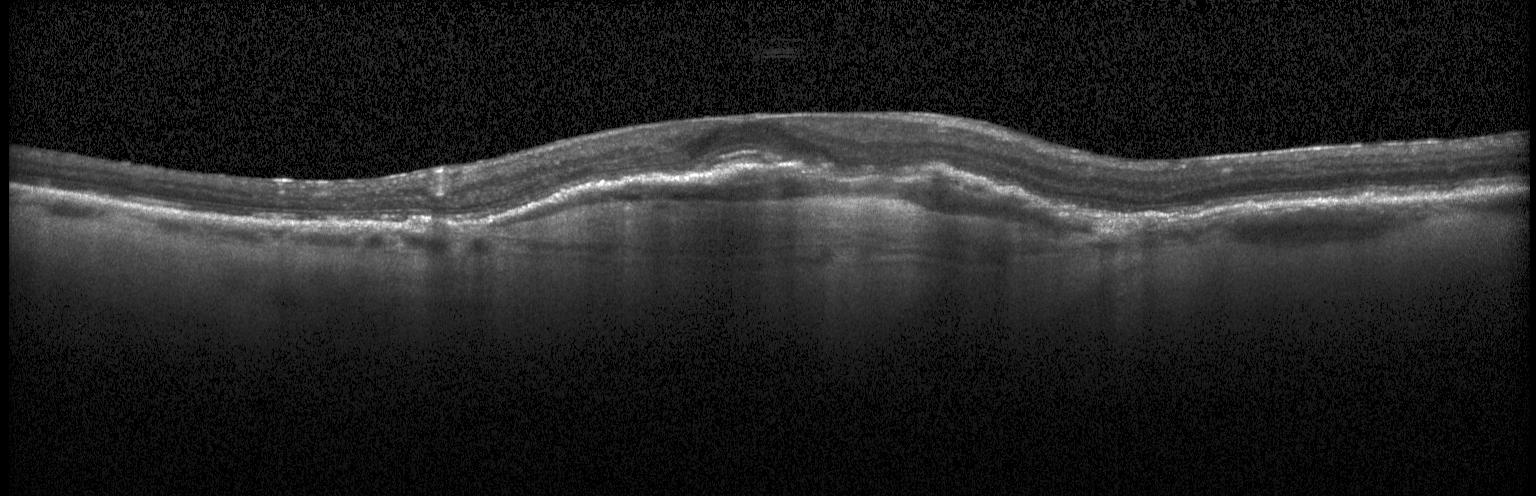

Macular OCT: choroidal neovascularization.